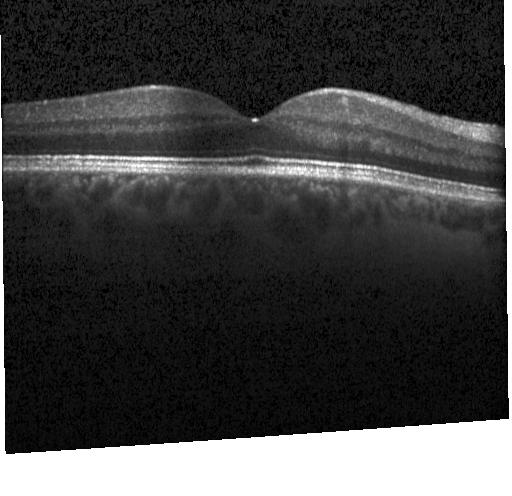

Retinal OCT B-scan
Dx: no evidence of choroidal neovascularization, diabetic macular edema, or drusen.